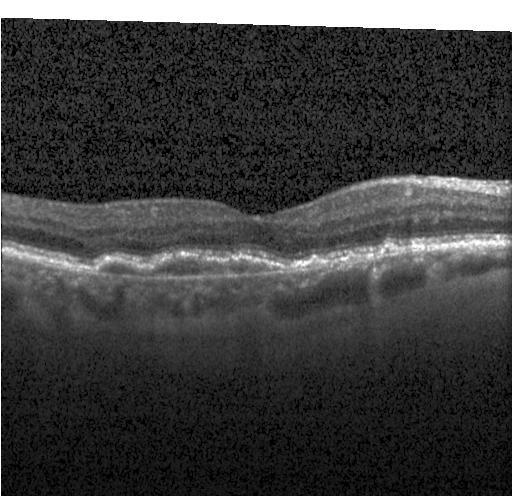

Spectral-domain optical coherence tomography, horizontal scan through the fovea, retinal OCT B-scan, Heidelberg Spectralis — This B-scan demonstrates choroidal neovascularization.